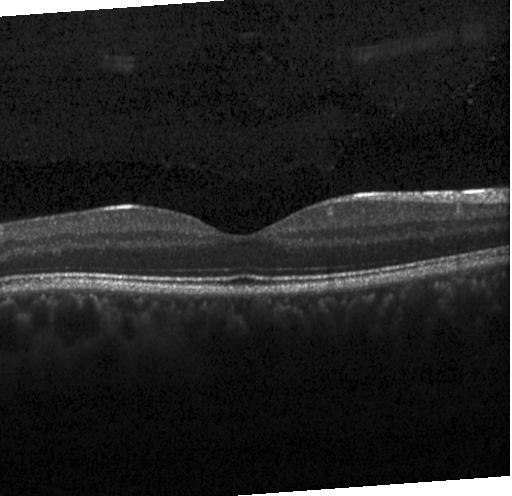 Retinal OCT cross-section showing no choroidal neovascularization, diabetic macular edema, or drusen.